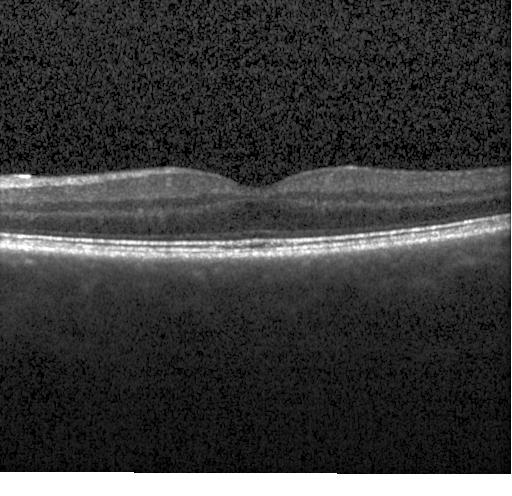

Diagnosis: no choroidal neovascularization, diabetic macular edema, or drusen.